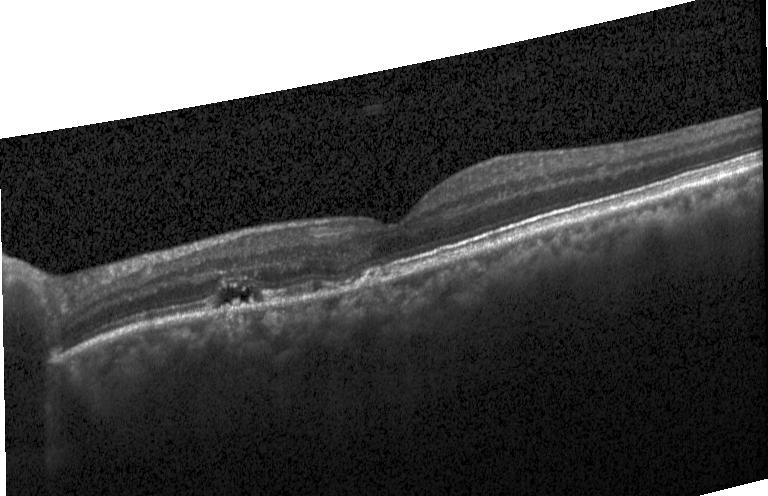 Optical coherence tomography scan — Choroidal neovascularization.